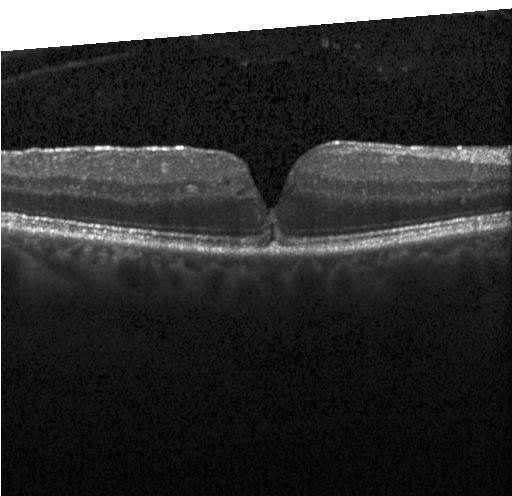

OCT B-scan showing diabetic macular edema (DME).